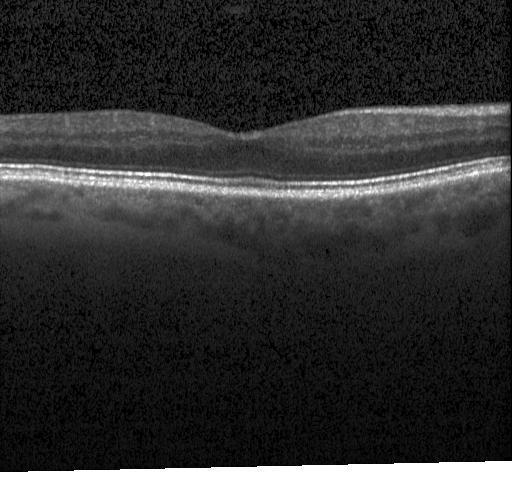
Fovea-centered · OCT line scan. The scan shows no choroidal neovascularization, no diabetic macular edema, and no drusen.